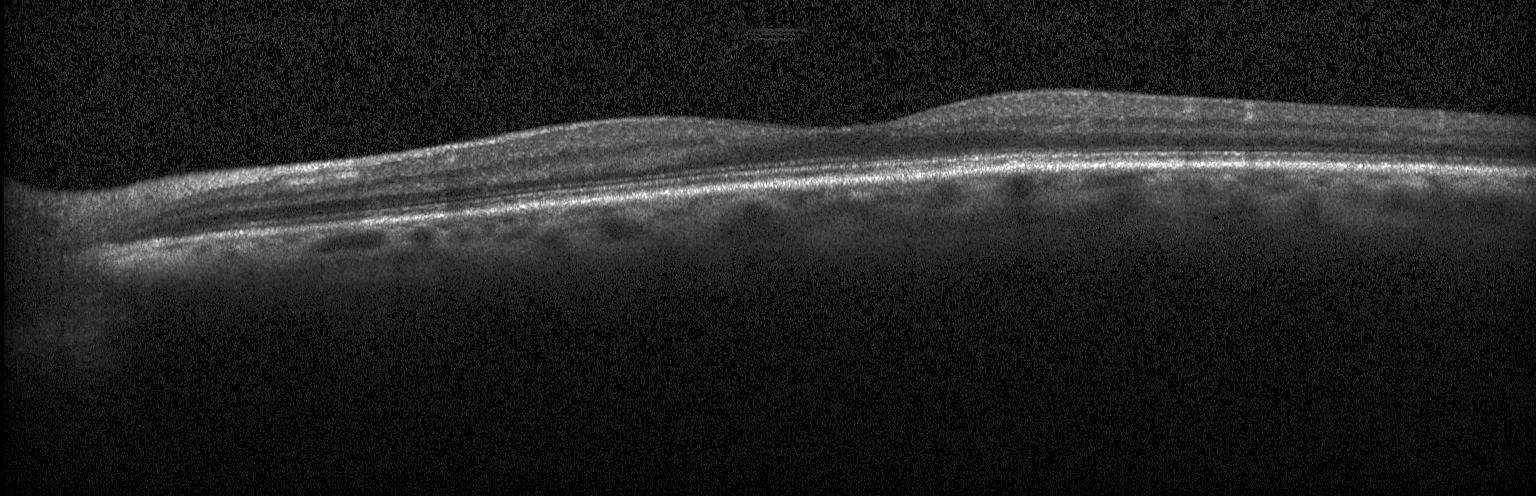

Heidelberg Spectralis OCT system. Retinal OCT B-scan. Through the macula. The scan shows neither choroidal neovascularization, diabetic macular edema, nor drusen.